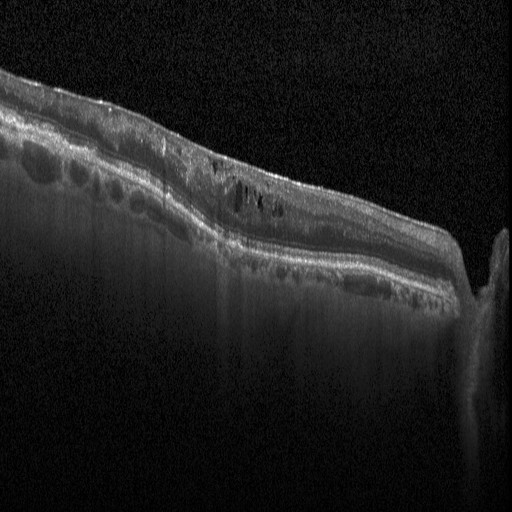

OCT B-scan · SD-OCT · instrument: Heidelberg Spectralis · through the macula. Diagnosis: DME.